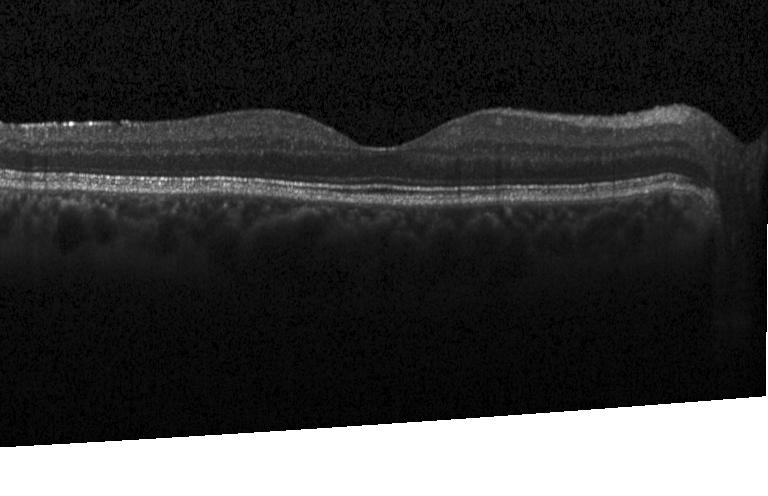

Spectral-domain optical coherence tomography, Heidelberg Spectralis, OCT B-scan
Impression: neither choroidal neovascularization, diabetic macular edema, nor drusen.